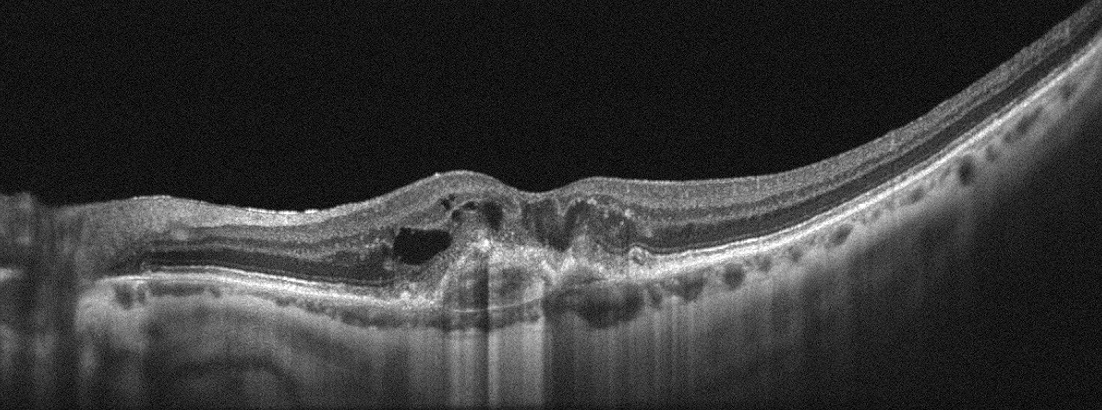
Retinal OCT cross-section; instrument: Optovue Avanti RTVue XR. Diagnosis: age-related macular degeneration (AMD).